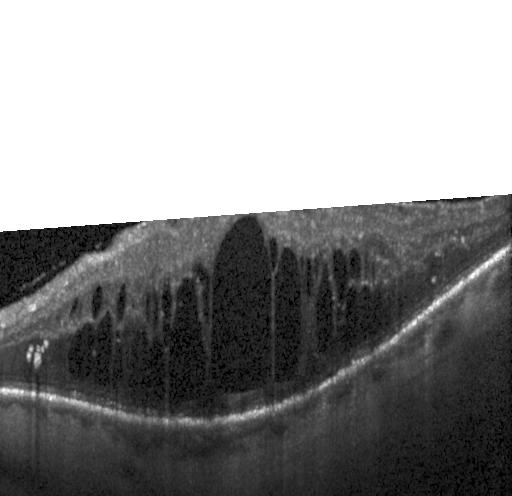 Spectral-domain OCT, fovea-centered, retinal OCT B-scan
Finding: DME.